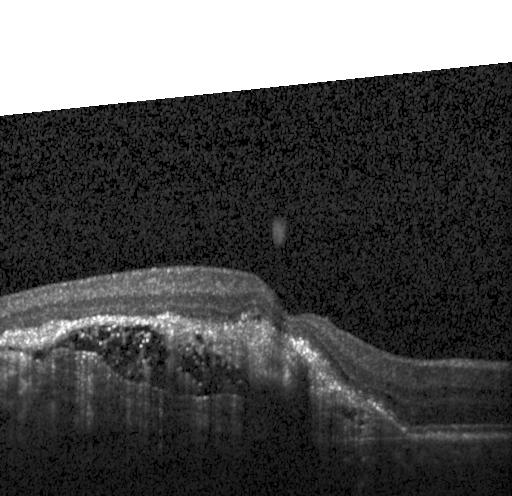 Acquired on a Heidelberg Spectralis · through the macula · SD-OCT · OCT B-scan.
Macular OCT: choroidal neovascularization.